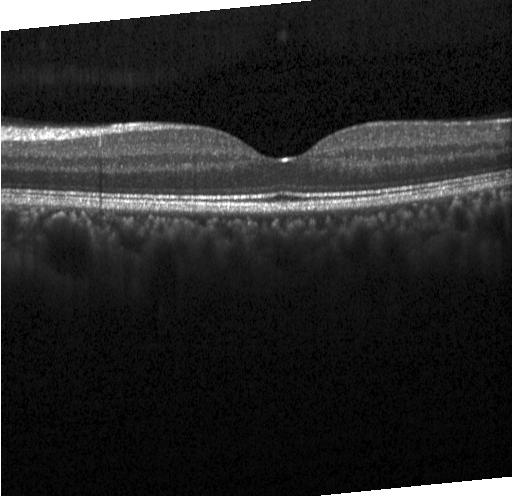 Diagnosis: no choroidal neovascularization, no diabetic macular edema, and no drusen.